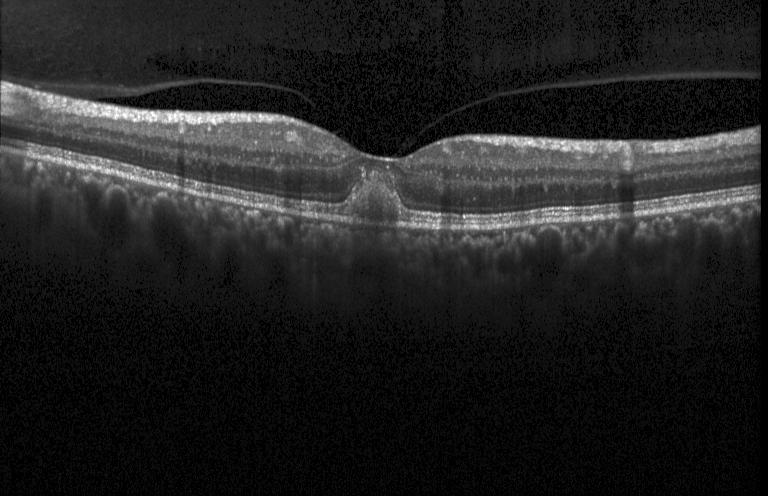
Retinal OCT cross-section showing choroidal neovascularization.